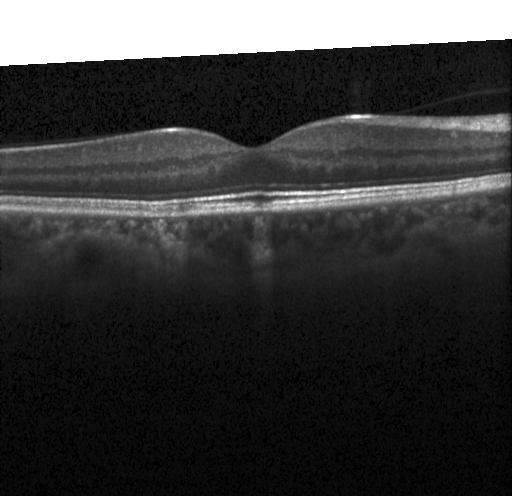 Fovea-centered; optical coherence tomography B-scan.
Assessment: neither choroidal neovascularization, diabetic macular edema, nor drusen.